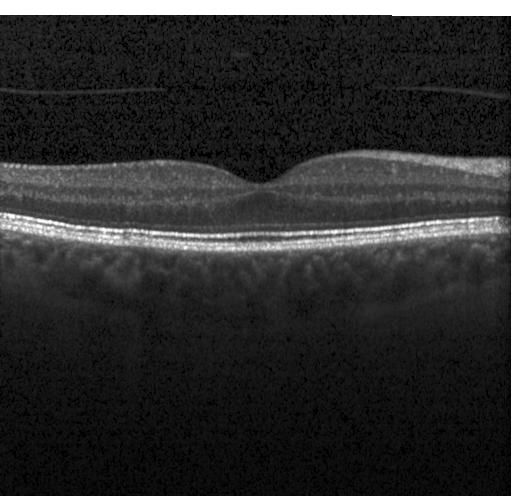
Diagnosis: no choroidal neovascularization, diabetic macular edema, or drusen.